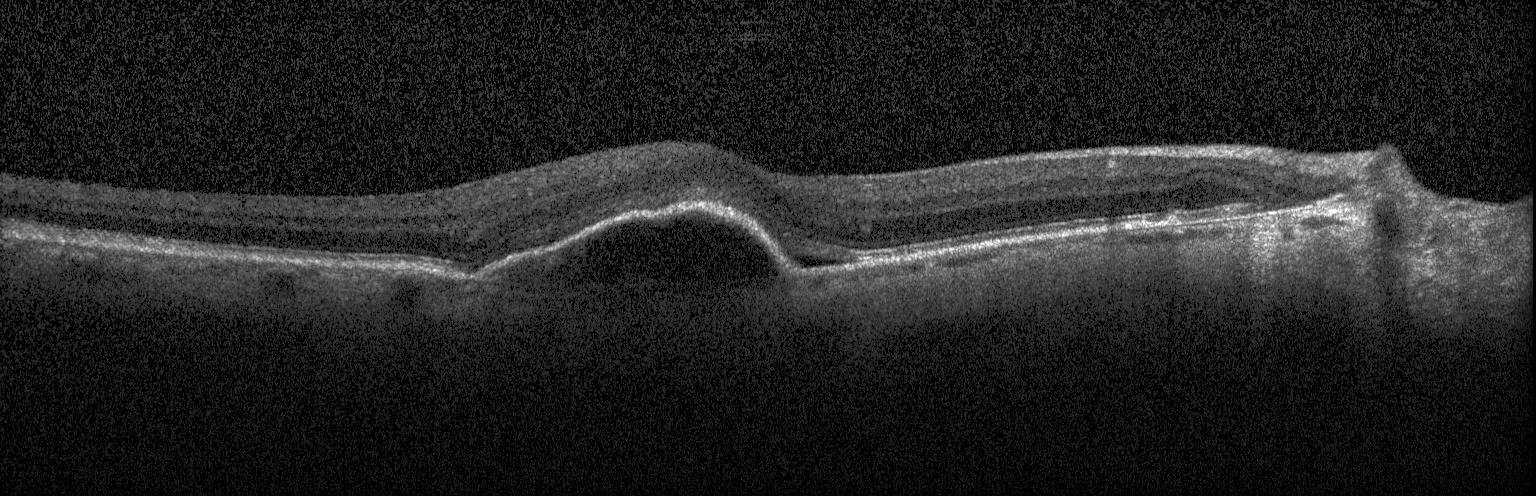 CNV.